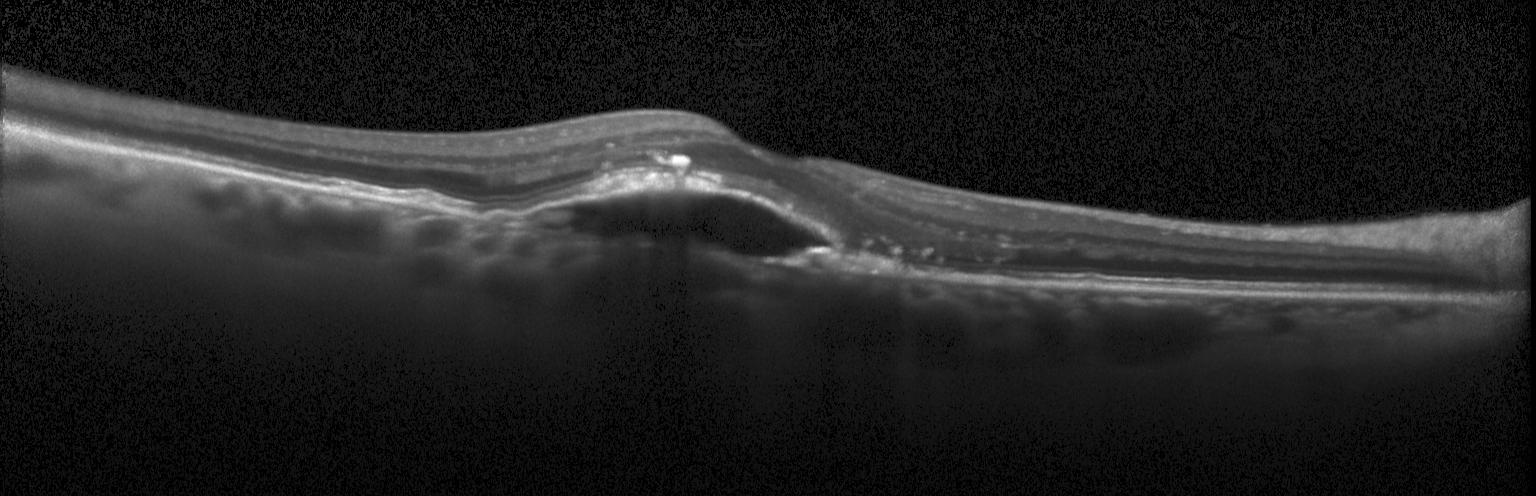
Diagnosis: choroidal neovascularization.